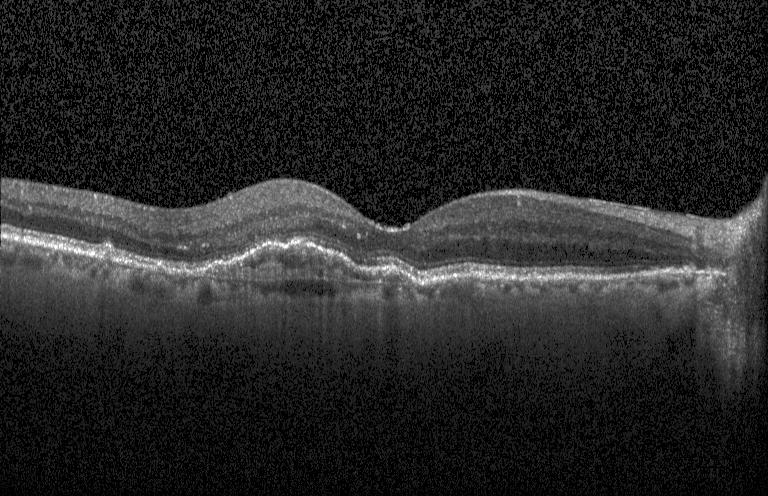
Spectral-domain optical coherence tomography. Retinal OCT cross-section. Finding: a choroidal neovascular membrane.